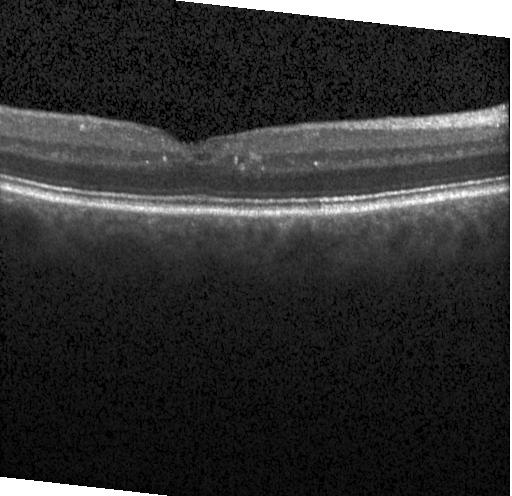 Retinal OCT cross-section — Assessment: no choroidal neovascularization, diabetic macular edema, or drusen.